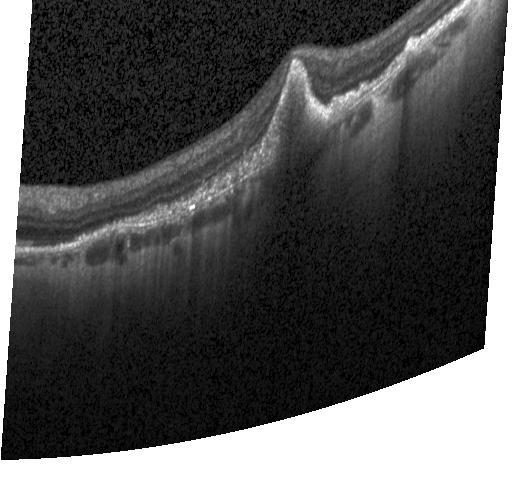
Assessment: CNV.